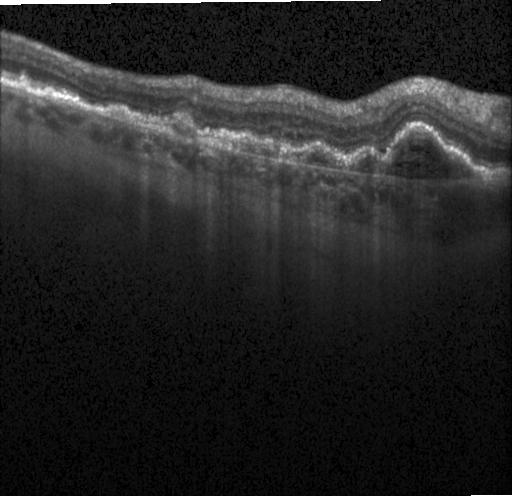
Heidelberg Spectralis, macular scan, spectral-domain OCT, optical coherence tomography B-scan. Choroidal neovascularization.